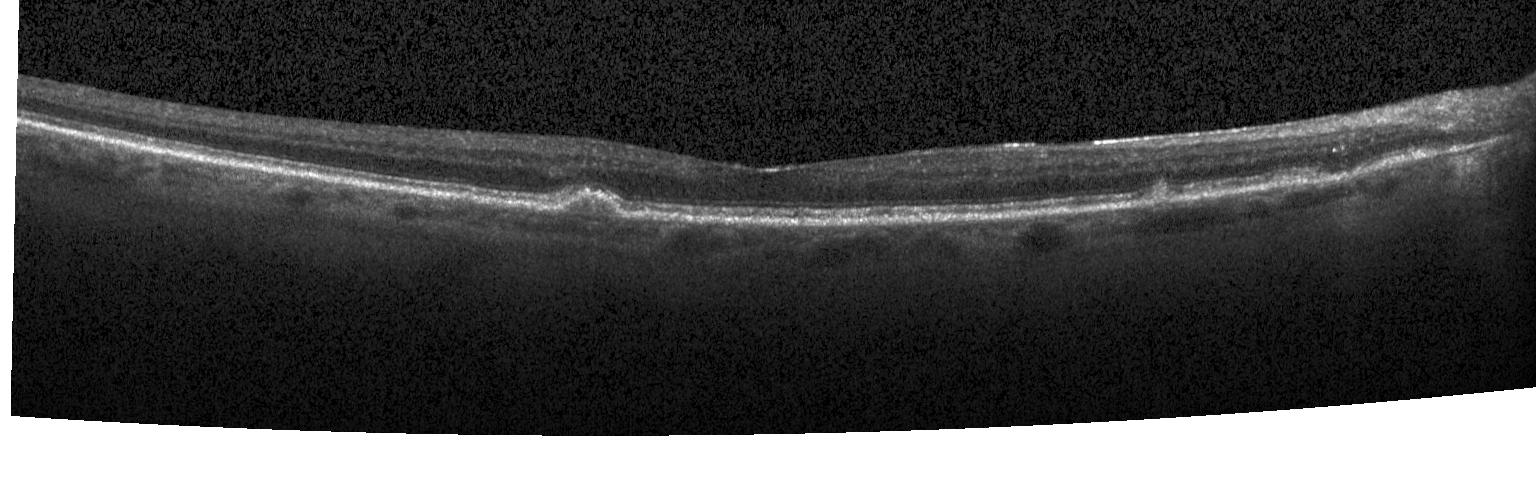

Retinal OCT B-scan. Assessment: sub-RPE drusenoid deposits.